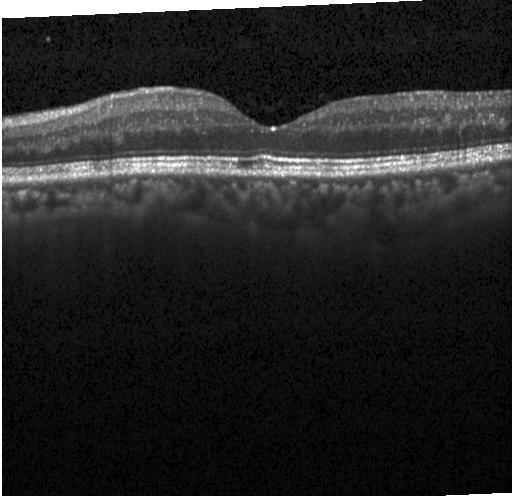 Retinal OCT B-scan.
Impression: no choroidal neovascularization, no diabetic macular edema, and no drusen.